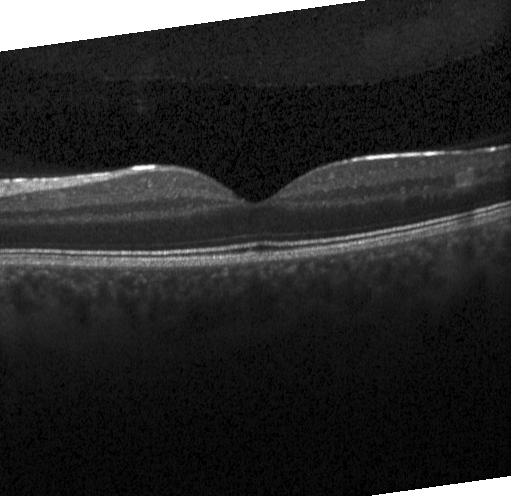

OCT finding: neither CNV, DME, nor drusen.